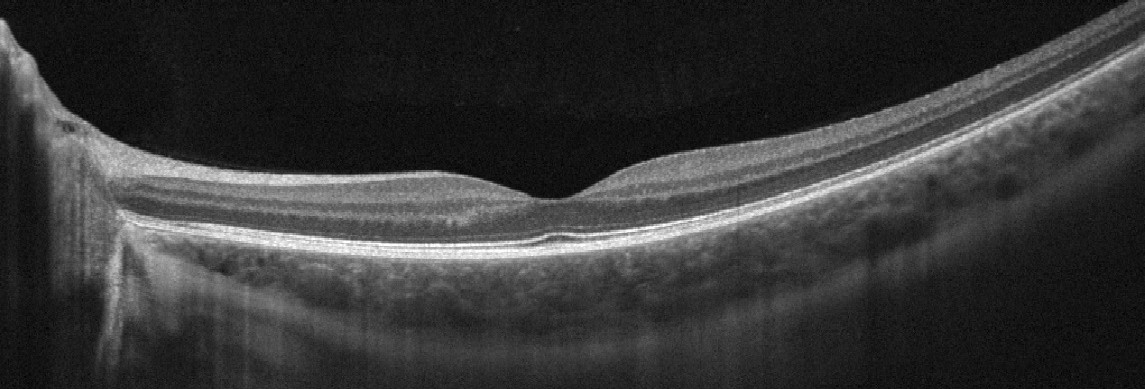 Retinal OCT cross-section — Diagnosis: no AMD, DME, ERM, RAO, RVO, or VID.